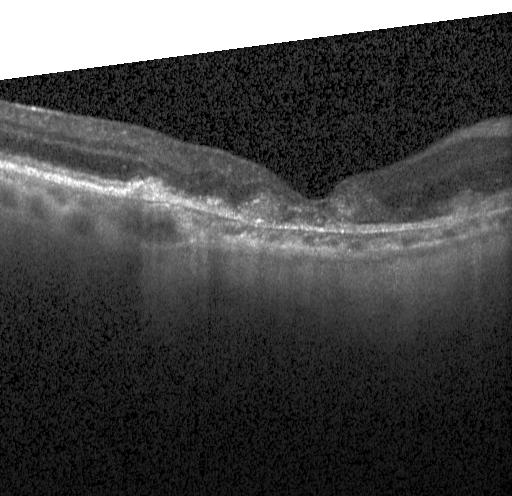 Spectral-domain OCT; retinal OCT B-scan. Finding: CNV.